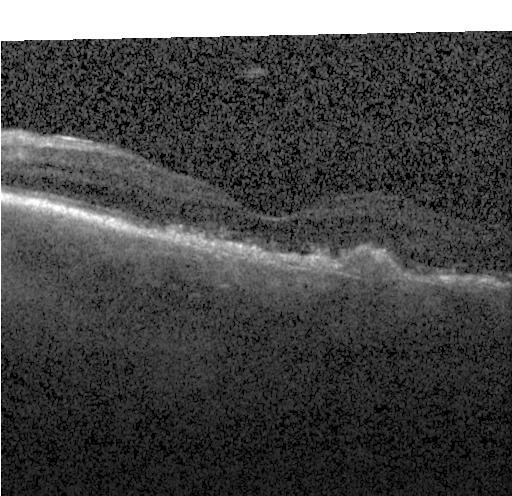

OCT B-scan. Heidelberg Spectralis. Macular scan. Spectral-domain optical coherence tomography
Impression: choroidal neovascularization (CNV).